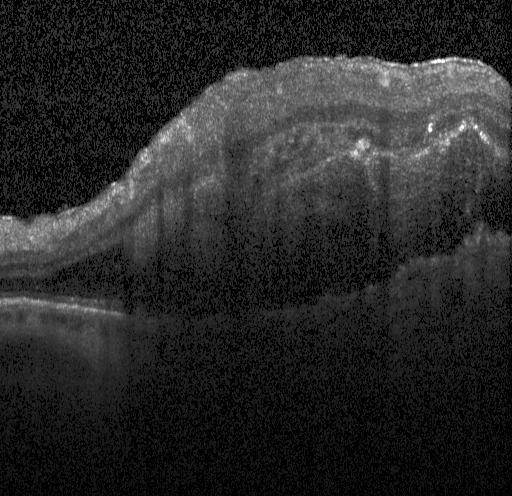

Through the macula · Heidelberg Spectralis · spectral-domain optical coherence tomography · retinal OCT B-scan — This B-scan demonstrates choroidal neovascularization (CNV).